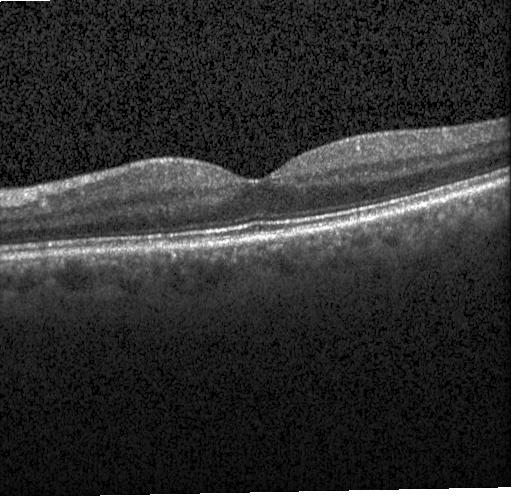
Retinal OCT B-scan
OCT finding: no choroidal neovascularization, no diabetic macular edema, and no drusen.